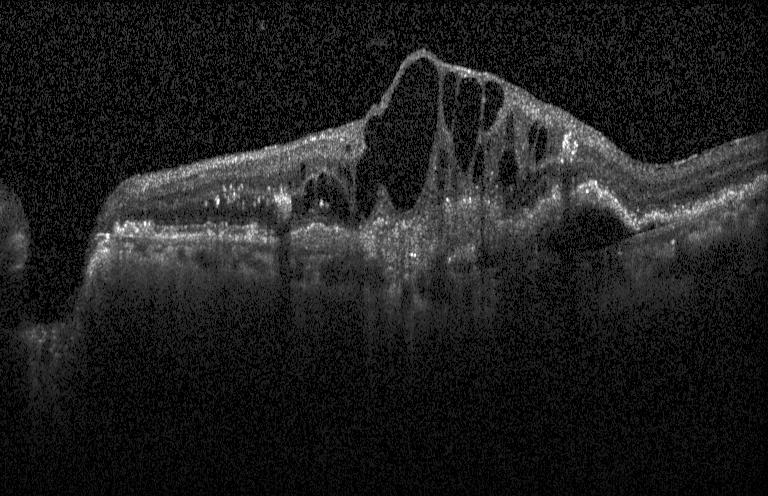
OCT B-scan — A choroidal neovascular membrane.